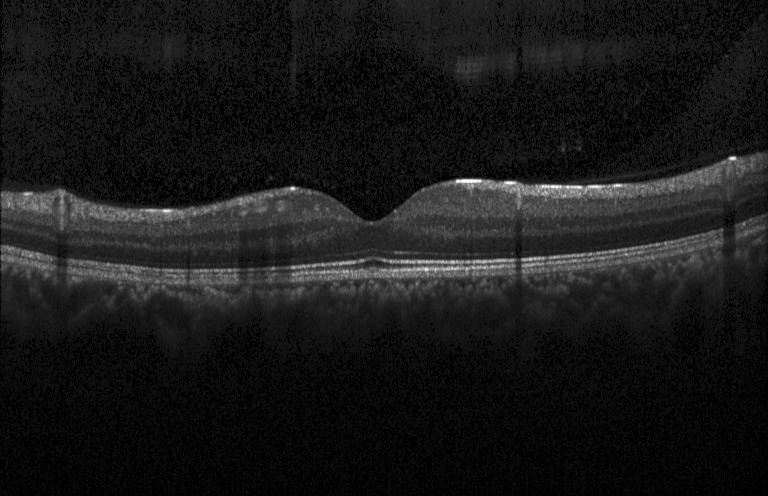

Neither choroidal neovascularization, diabetic macular edema, nor drusen.